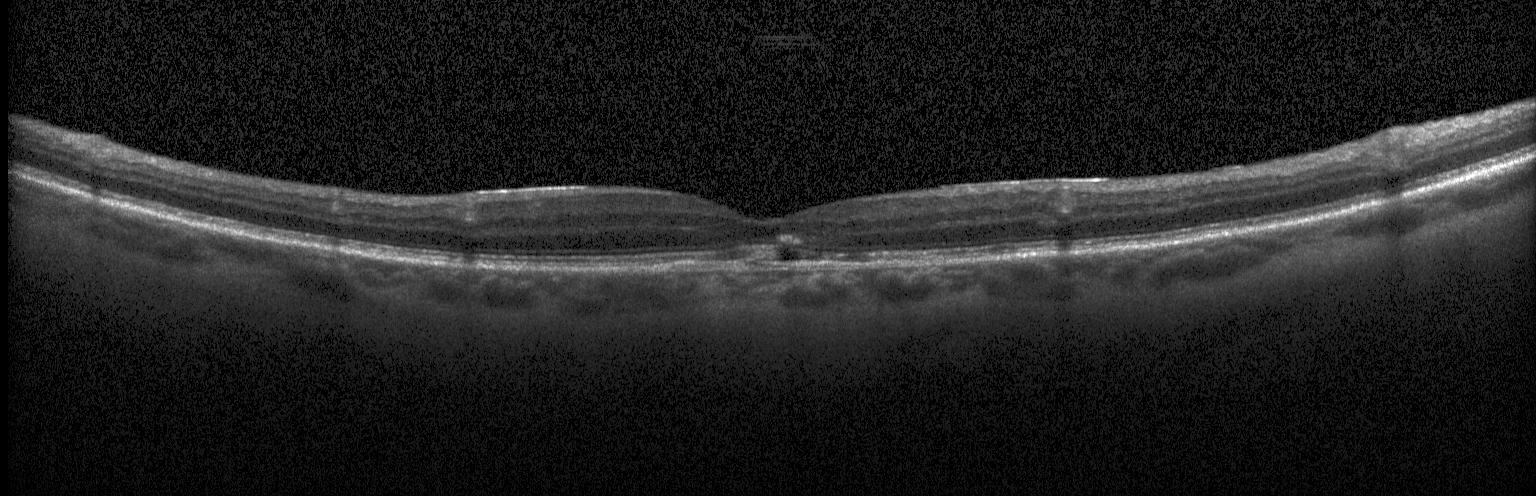 Spectral-domain OCT; OCT B-scan; acquired on a Heidelberg Spectralis; fovea-centered.
Dx: a choroidal neovascular membrane.